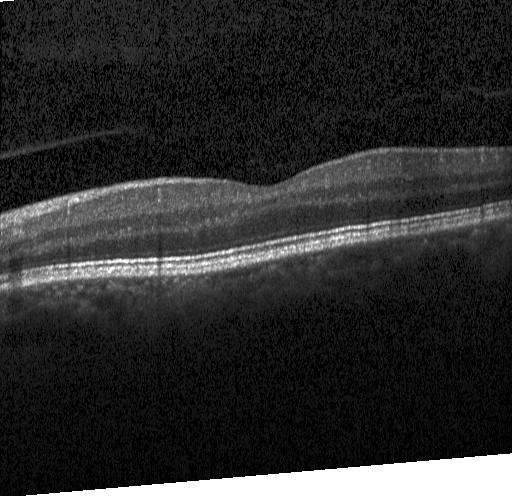
Heidelberg Spectralis; SD-OCT; optical coherence tomography B-scan. Neither CNV, DME, nor drusen.